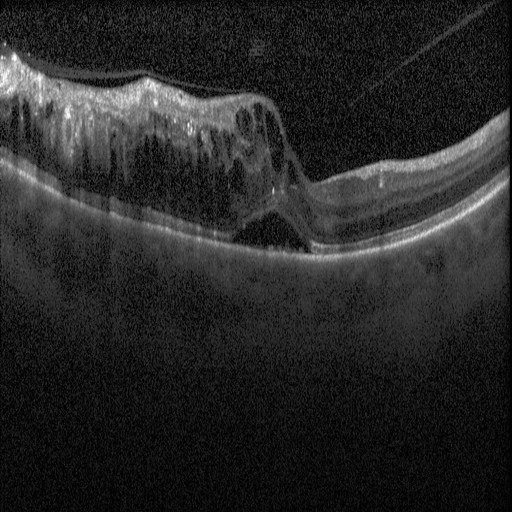

OCT B-scan. Finding: diabetic macular edema (DME).